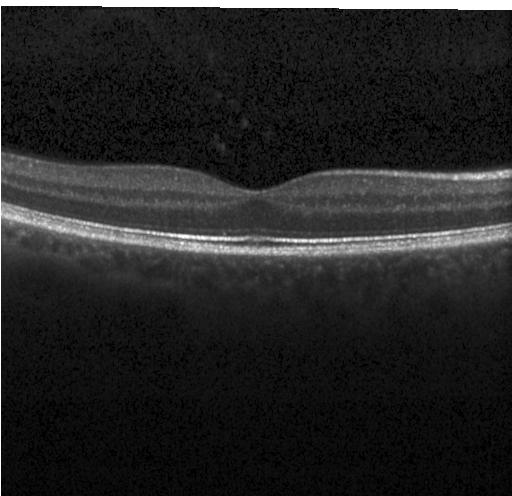 Finding: no choroidal neovascularization, diabetic macular edema, or drusen.